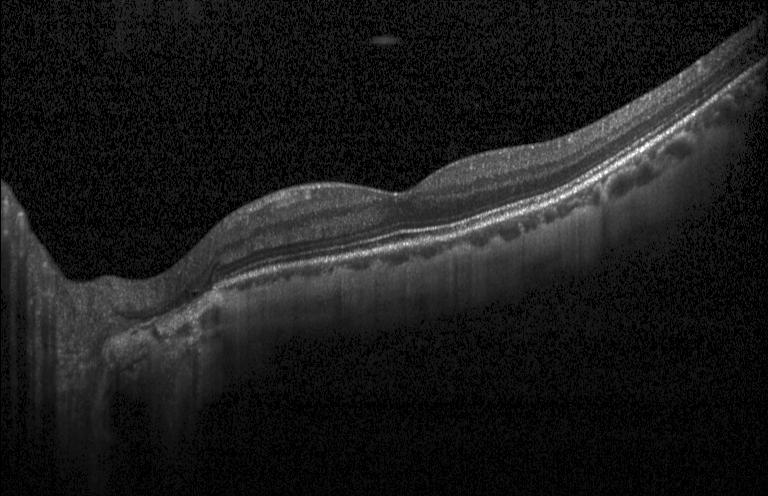 Optical coherence tomography B-scan — No evidence of choroidal neovascularization, diabetic macular edema, or drusen.